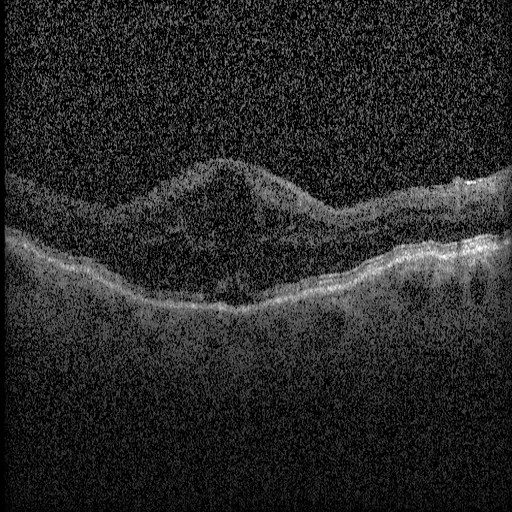 Acquired on a Heidelberg Spectralis. Retinal OCT B-scan — Impression: diabetic macular edema.